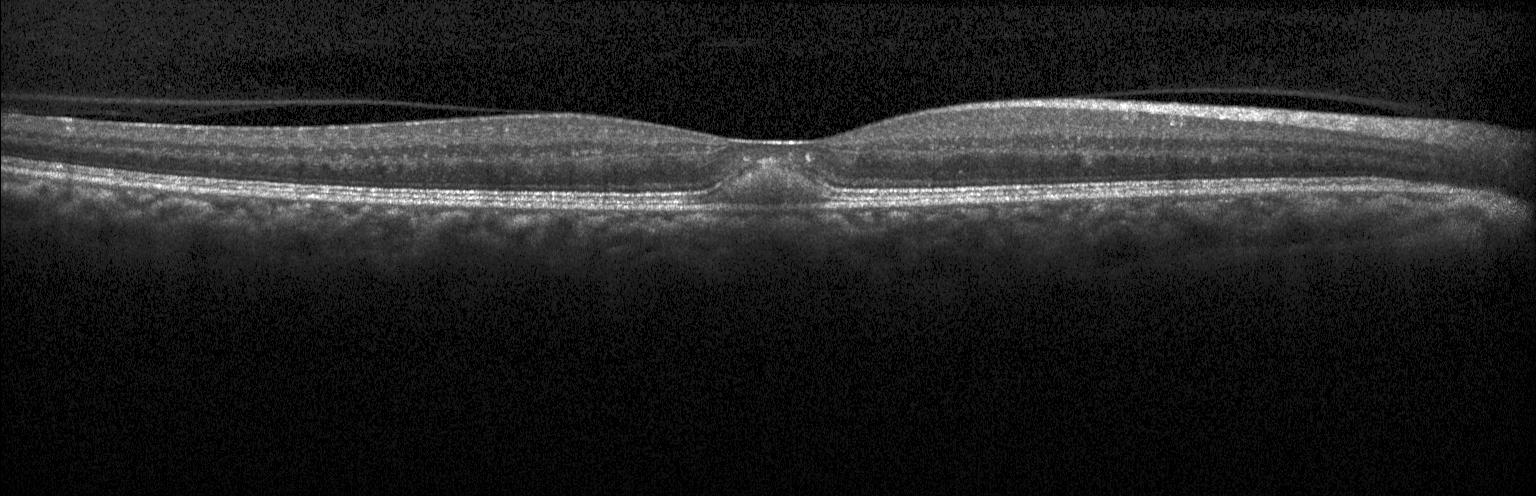
Retinal OCT cross-section showing choroidal neovascularization (CNV).